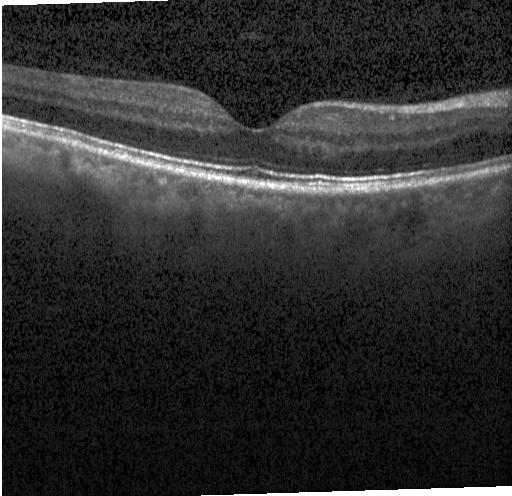
Spectral-domain optical coherence tomography, retinal OCT cross-section, Heidelberg Spectralis OCT system.
Impression: neither choroidal neovascularization, diabetic macular edema, nor drusen.